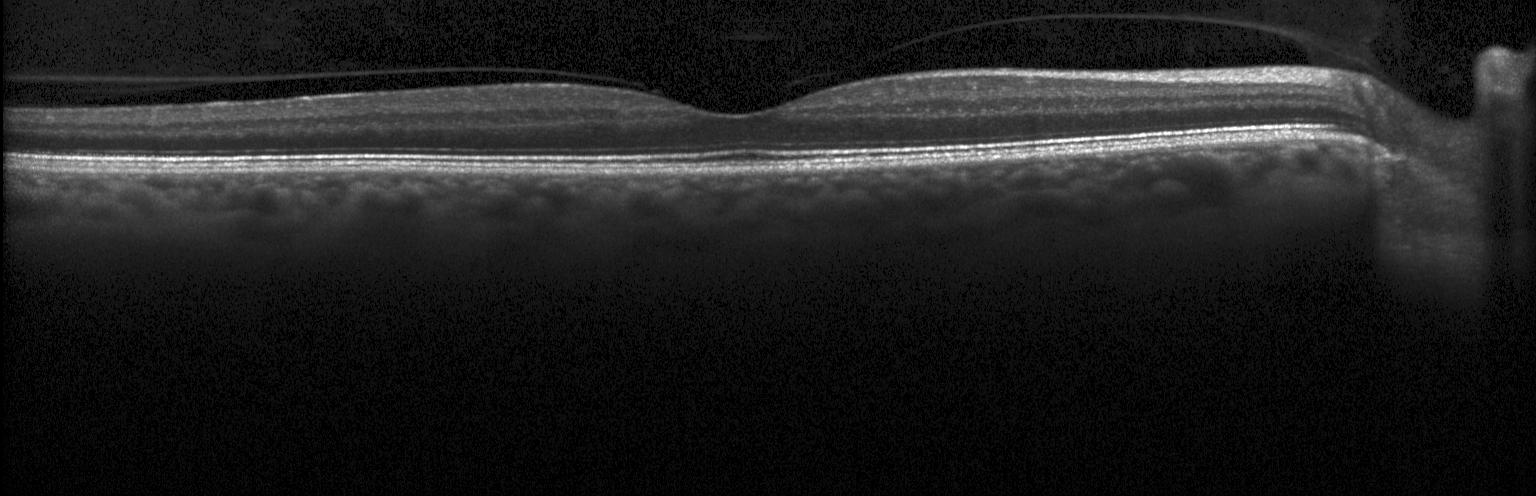
Assessment: neither choroidal neovascularization, diabetic macular edema, nor drusen.